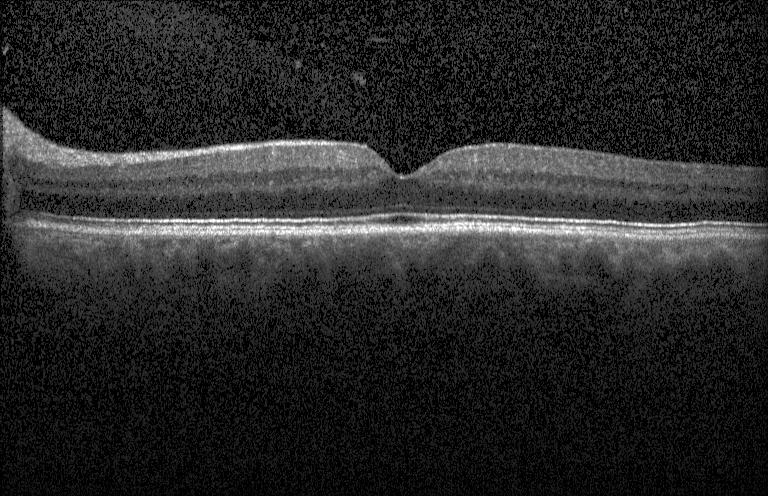

Dx: no evidence of choroidal neovascularization, diabetic macular edema, or drusen.